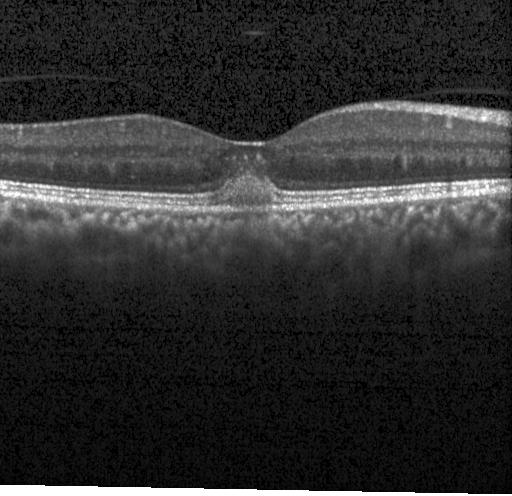

Impression: CNV.